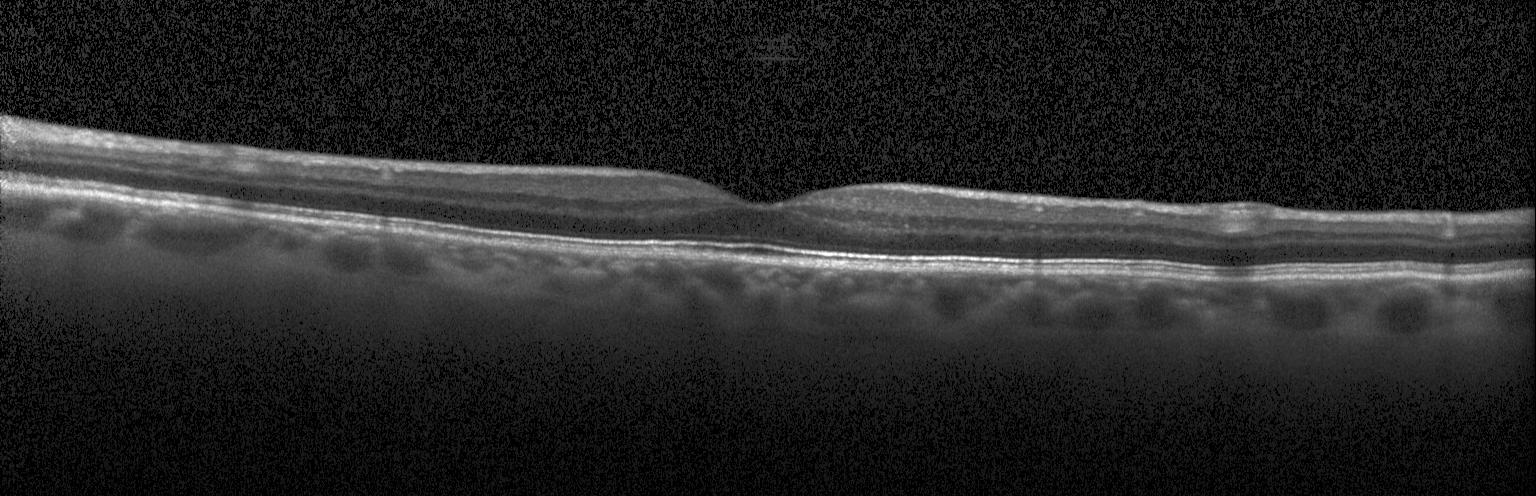
Finding: no choroidal neovascularization, diabetic macular edema, or drusen.